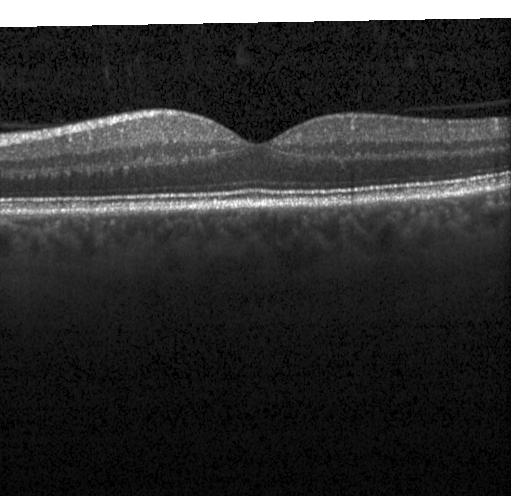

Impression: neither CNV, DME, nor drusen.